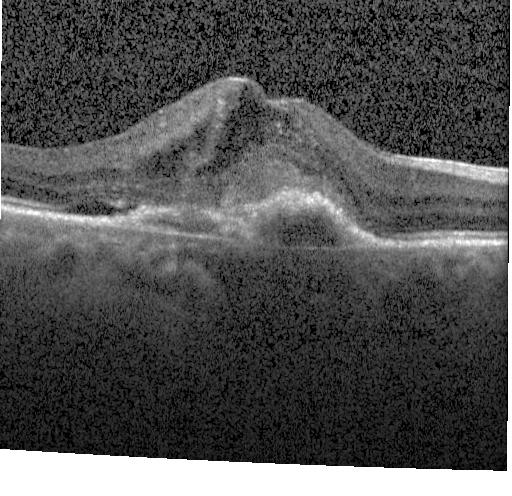

OCT B-scan, through the macula, SD-OCT. Impression: a choroidal neovascular membrane.